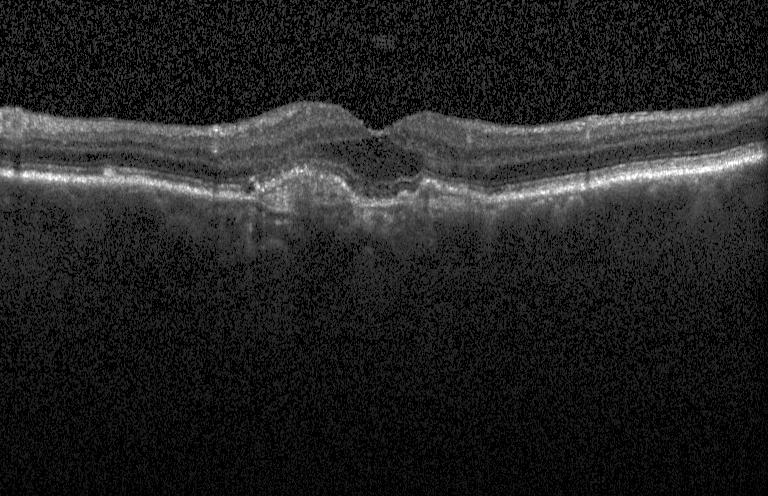
Impression: choroidal neovascularization.